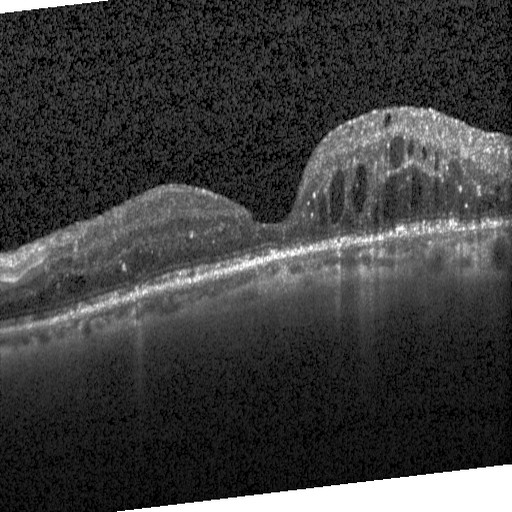

Retinal OCT cross-section showing diabetic macular edema.